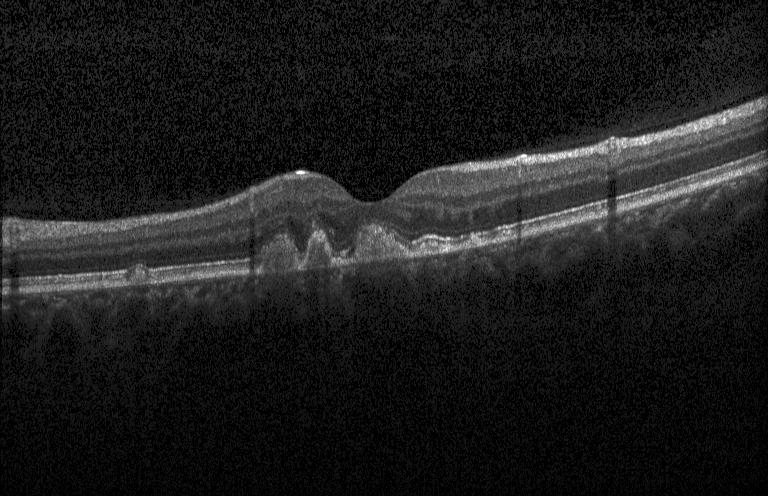

Spectral-domain OCT. Centered on the fovea. Acquired on a Heidelberg Spectralis. OCT B-scan — Finding: multiple drusen.